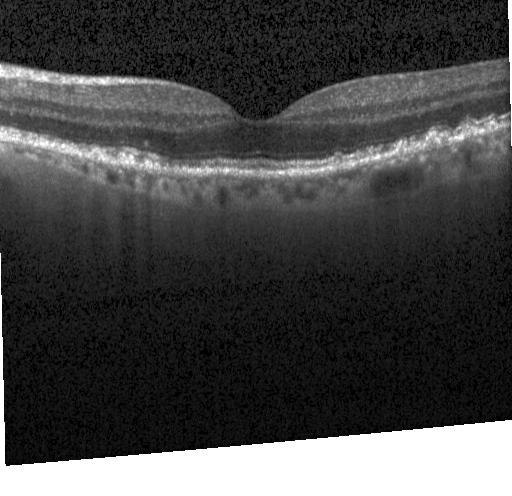

Spectral-domain OCT B-scan: multiple drusen.